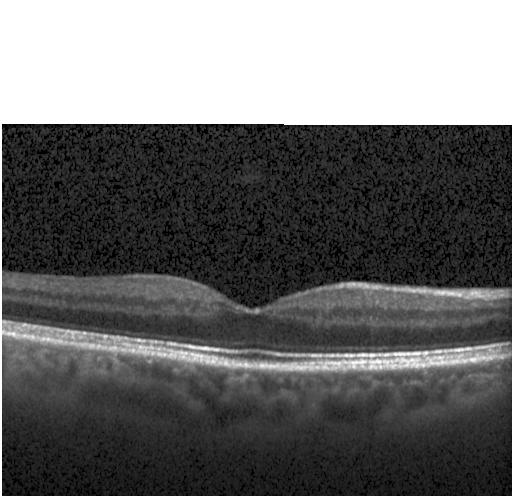

Optical coherence tomography B-scan.
Impression: no choroidal neovascularization, diabetic macular edema, or drusen.